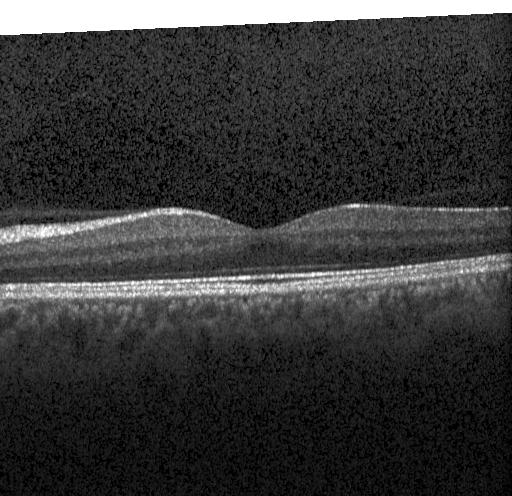

Impression: no choroidal neovascularization, no diabetic macular edema, and no drusen.